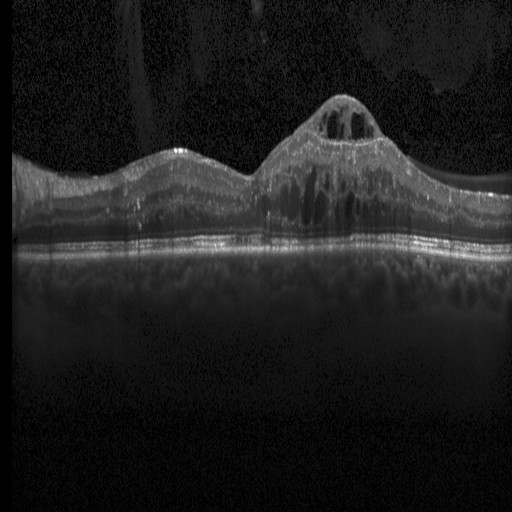
Assessment: diabetic macular edema (DME).